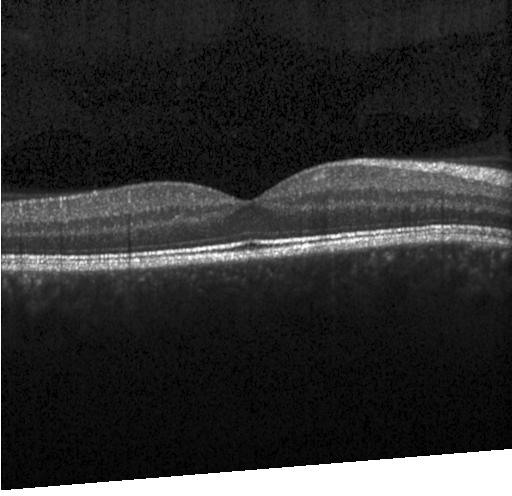
Retinal OCT cross-section — Diagnosis: no choroidal neovascularization, diabetic macular edema, or drusen.